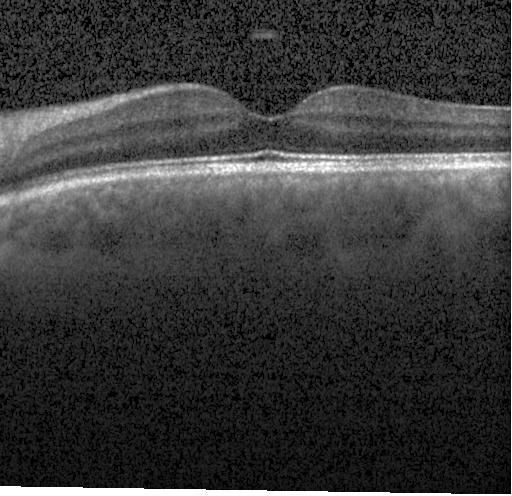
Spectral-domain OCT B-scan: no choroidal neovascularization, no diabetic macular edema, and no drusen.